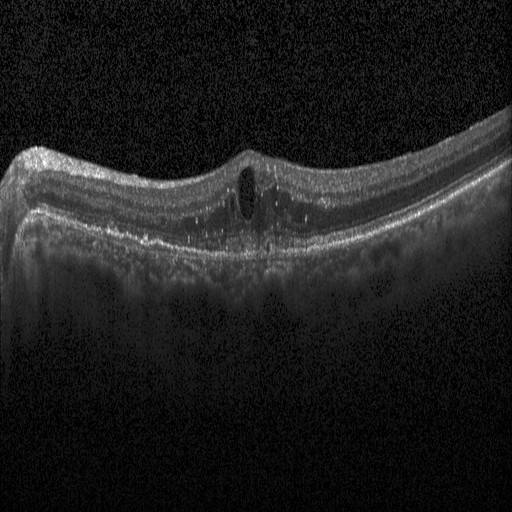

Through the macula · retinal OCT cross-section · SD-OCT · instrument: Heidelberg Spectralis — Finding: DME.